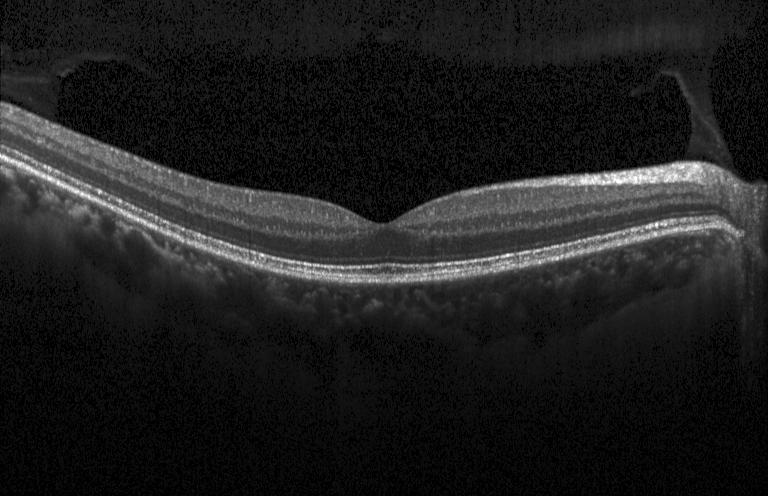 OCT line scan
Macular OCT: no choroidal neovascularization, diabetic macular edema, or drusen.